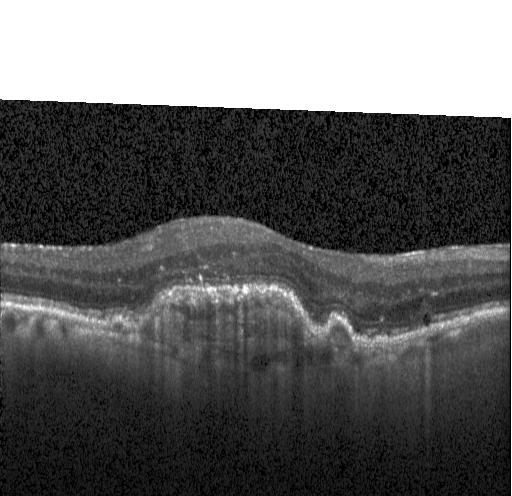 This B-scan demonstrates a choroidal neovascular membrane.